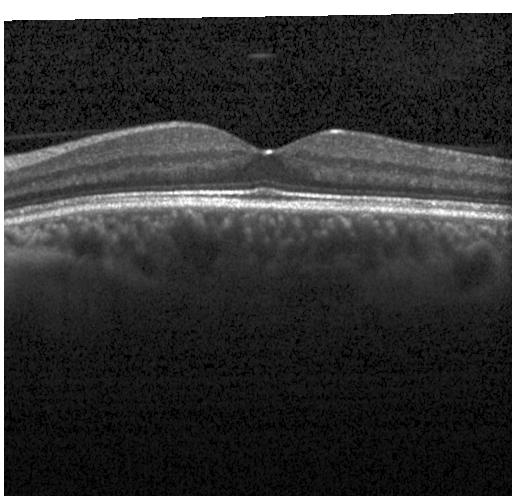
Retinal OCT B-scan.
Finding: no choroidal neovascularization, diabetic macular edema, or drusen.